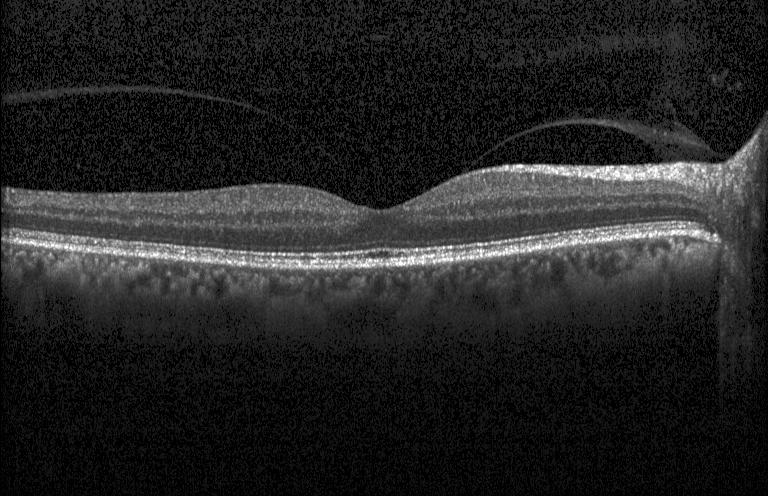 Dx: no evidence of choroidal neovascularization, diabetic macular edema, or drusen.